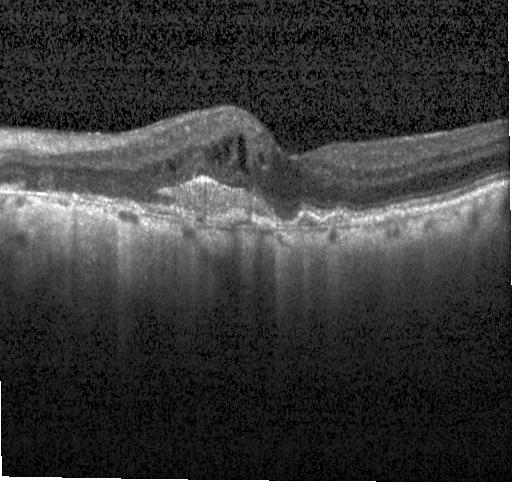

Heidelberg Spectralis OCT system. Spectral-domain optical coherence tomography. Optical coherence tomography B-scan. Horizontal scan through the fovea — This B-scan demonstrates a choroidal neovascular membrane.